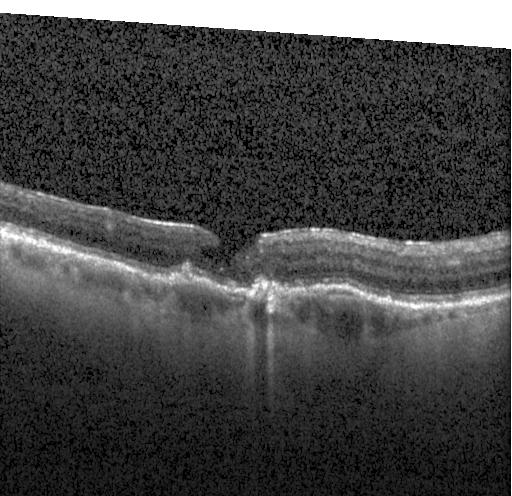
Finding: a choroidal neovascular membrane.